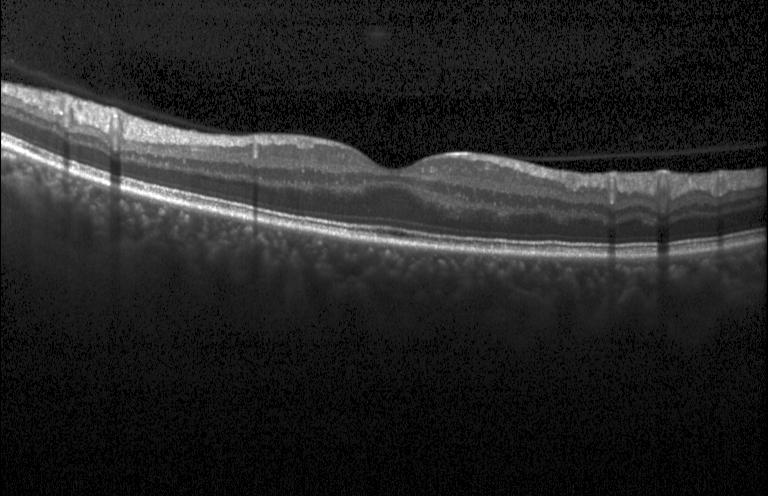

SD-OCT. OCT B-scan. Macular scan. Acquired on a Heidelberg Spectralis
Finding: no choroidal neovascularization, no diabetic macular edema, and no drusen.